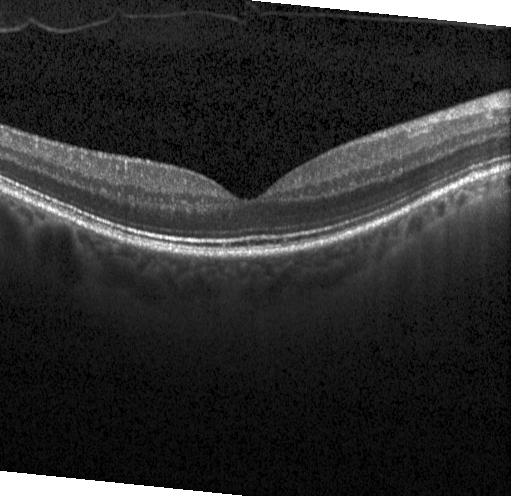
Acquired on a Heidelberg Spectralis · macular scan · OCT B-scan.
Assessment: no choroidal neovascularization, no diabetic macular edema, and no drusen.